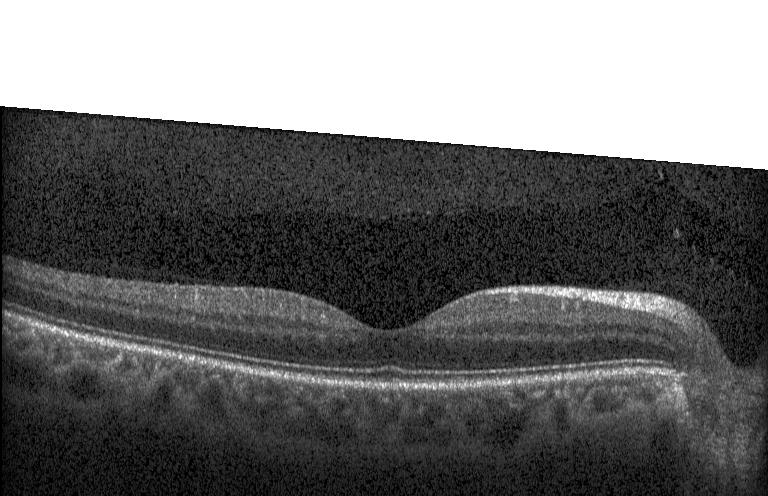
Through the macula · optical coherence tomography scan.
No choroidal neovascularization, diabetic macular edema, or drusen.